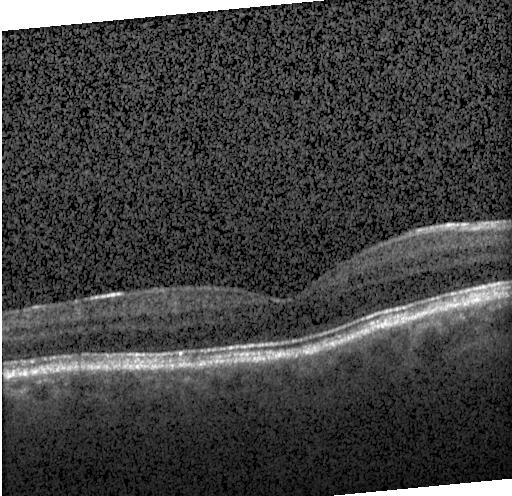

Optical coherence tomography B-scan. Instrument: Heidelberg Spectralis. Diagnosis: no evidence of CNV, DME, or drusen.